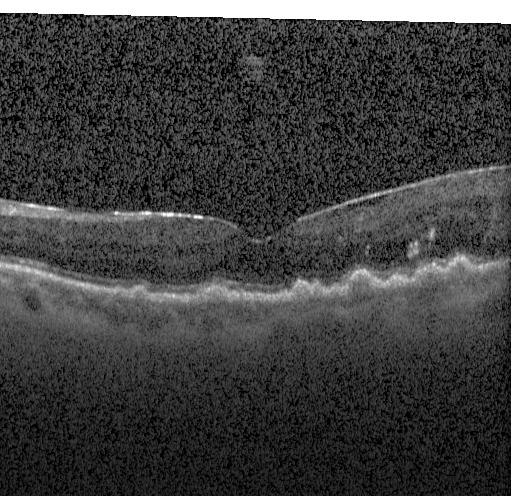 Assessment: multiple drusen.